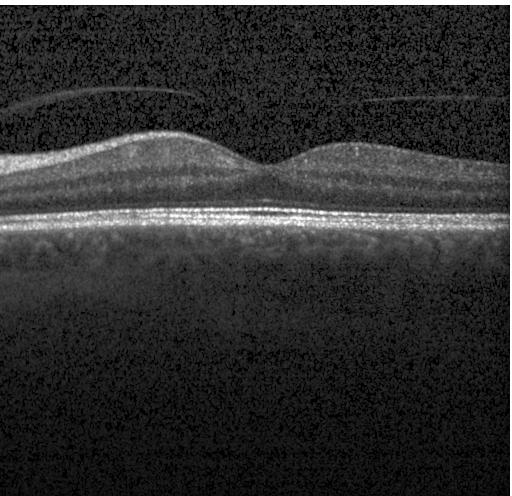

Spectral-domain optical coherence tomography, OCT line scan, horizontal scan through the fovea. OCT finding: neither choroidal neovascularization, diabetic macular edema, nor drusen.